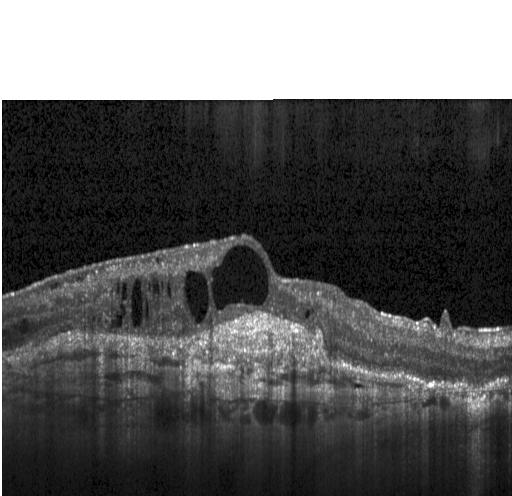 Spectral-domain optical coherence tomography; through the macula; optical coherence tomography B-scan; Heidelberg Spectralis. Impression: a choroidal neovascular membrane.